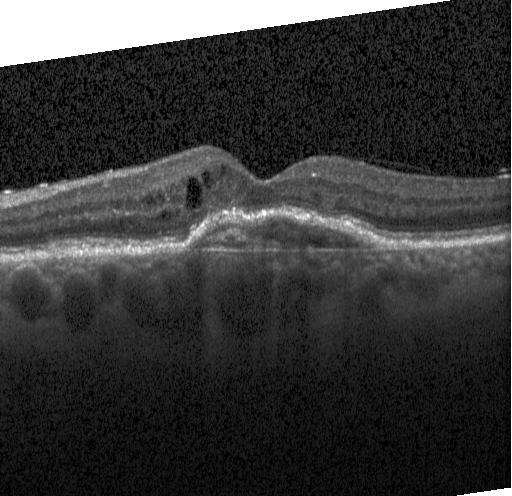
Retinal OCT B-scan.
Macular OCT: a choroidal neovascular membrane.